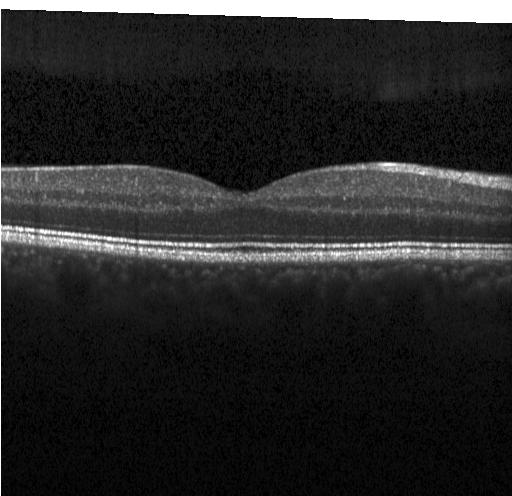 OCT B-scan showing no choroidal neovascularization, no diabetic macular edema, and no drusen.